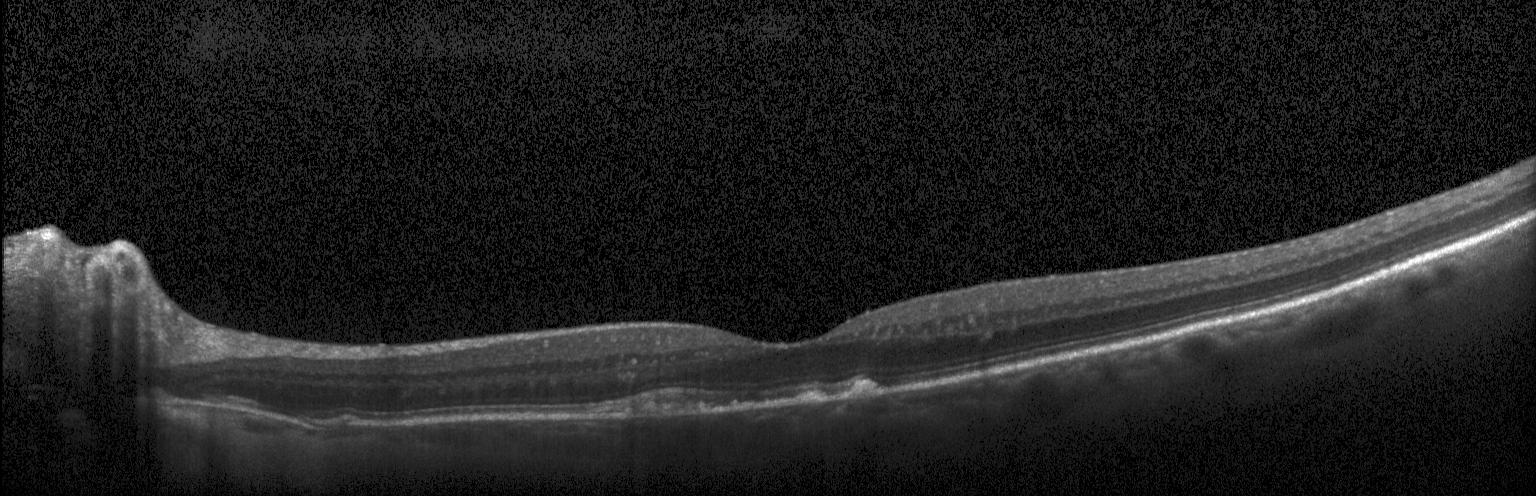
SD-OCT · OCT B-scan · Heidelberg Spectralis
This B-scan demonstrates multiple drusen.